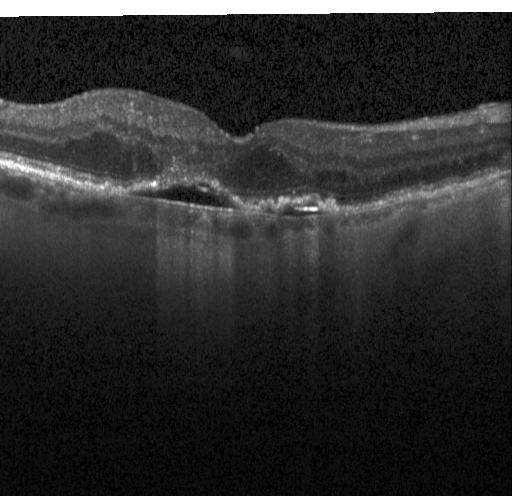
Impression: a choroidal neovascular membrane.